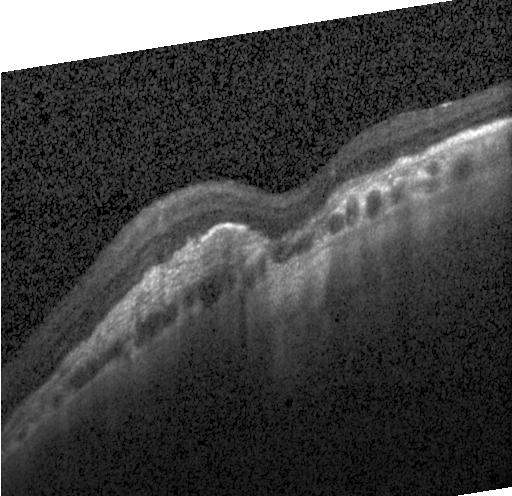
Retinal OCT B-scan. Heidelberg Spectralis OCT system. SD-OCT — Diagnosis: CNV.